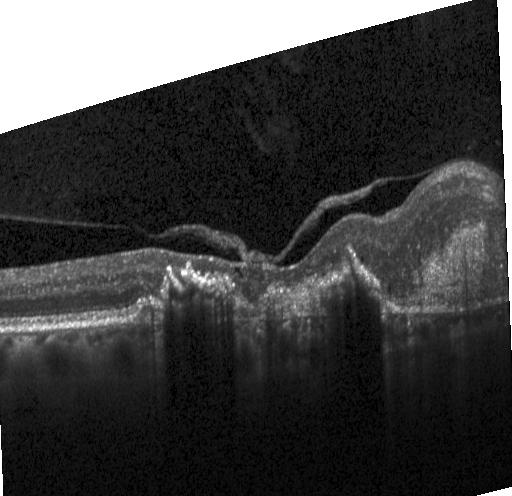
The scan shows choroidal neovascularization.